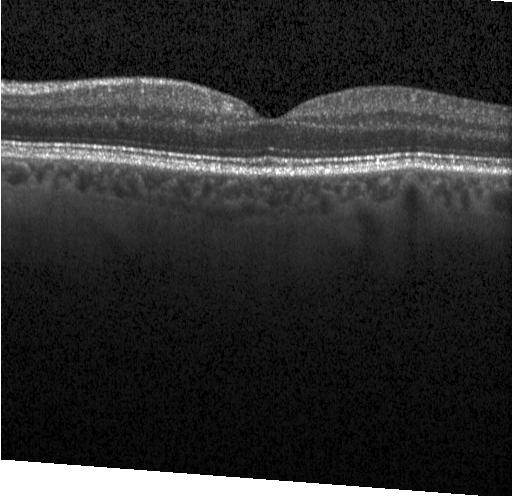
Retinal OCT B-scan
Assessment: neither choroidal neovascularization, diabetic macular edema, nor drusen.